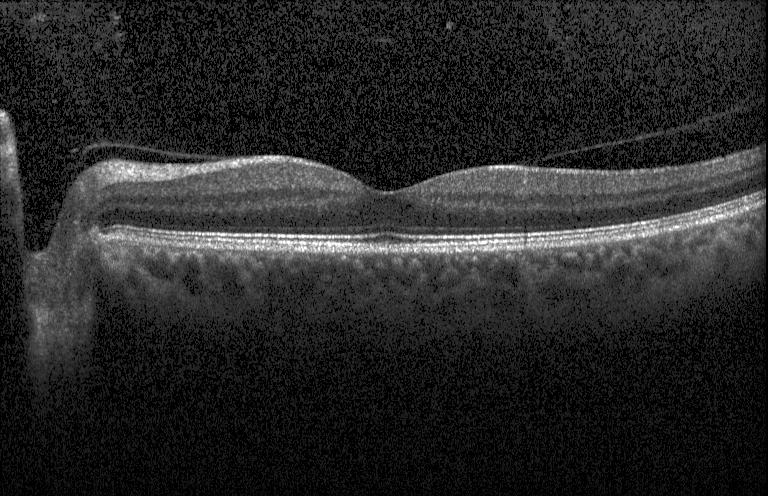
Retinal OCT B-scan. SD-OCT. Instrument: Heidelberg Spectralis
No CNV, no DME, and no drusen.